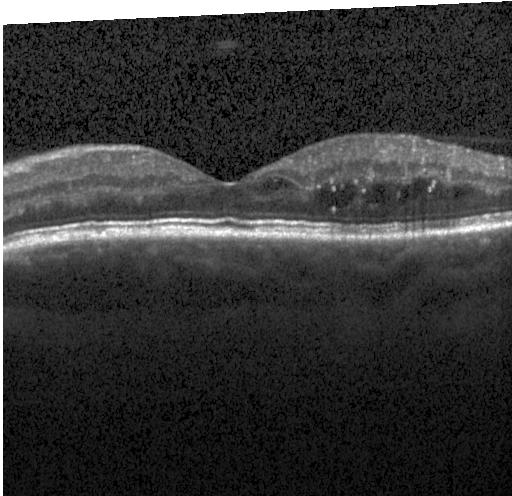
Retinal OCT B-scan.
DME.